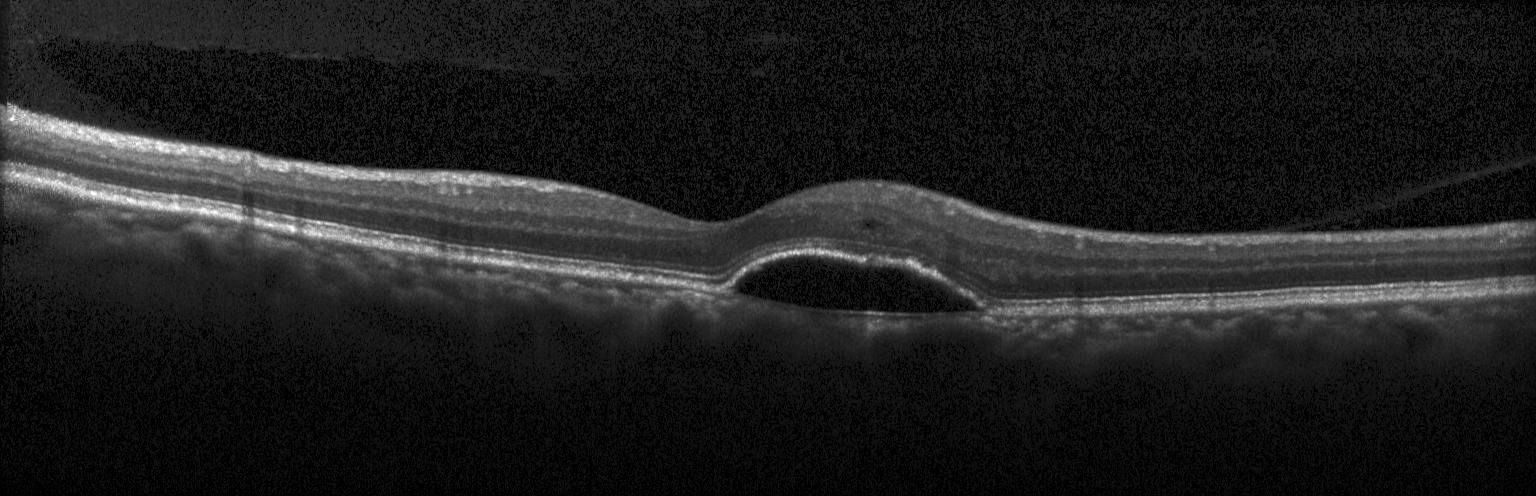 CNV.